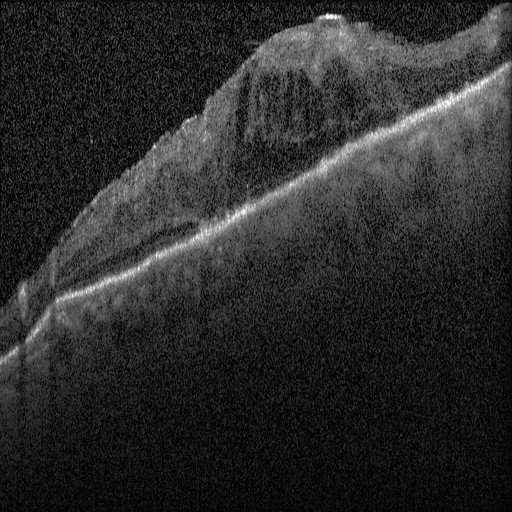

OCT finding: diabetic macular edema.